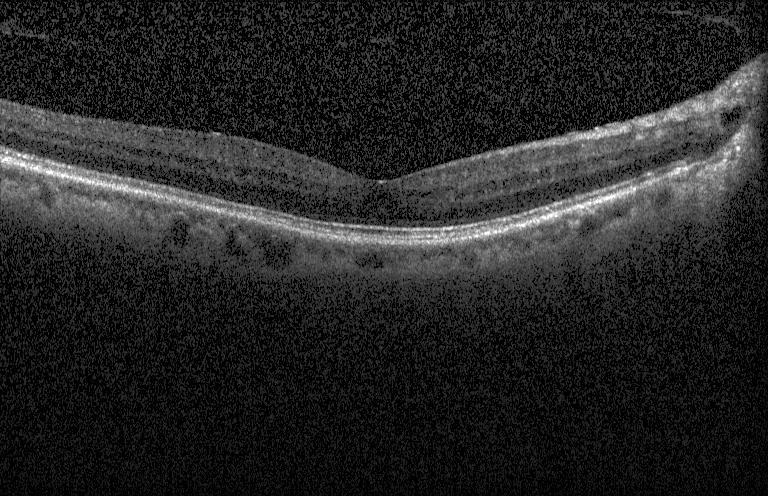 Through the macula · spectral-domain OCT · retinal OCT B-scan
Assessment: no evidence of choroidal neovascularization, diabetic macular edema, or drusen.